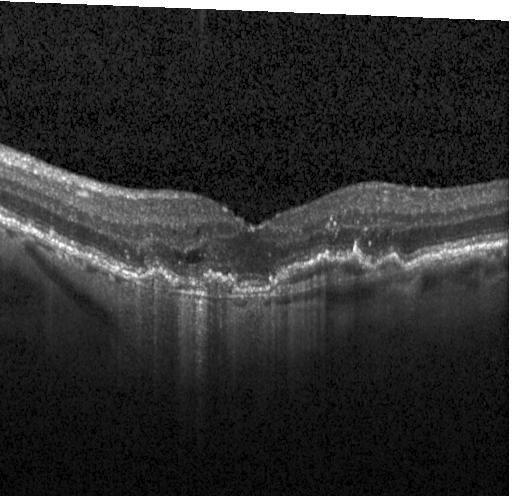 Spectral-domain optical coherence tomography, retinal OCT cross-section, instrument: Heidelberg Spectralis — Finding: choroidal neovascularization.